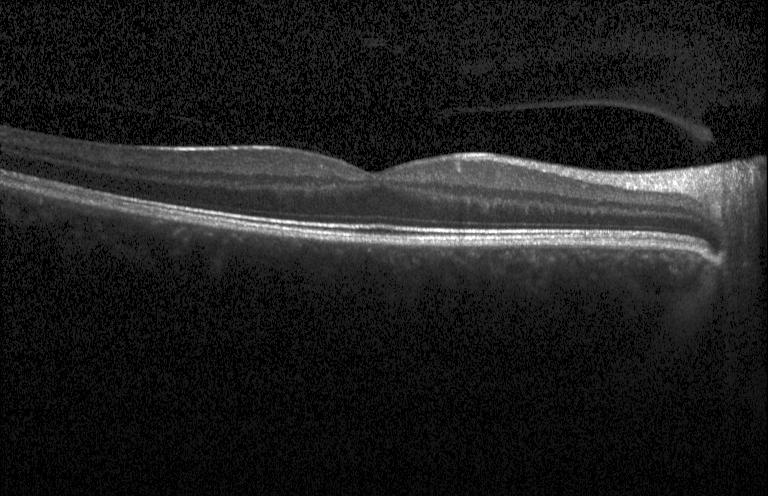
Heidelberg Spectralis, retinal OCT B-scan, spectral-domain OCT — Neither CNV, DME, nor drusen.